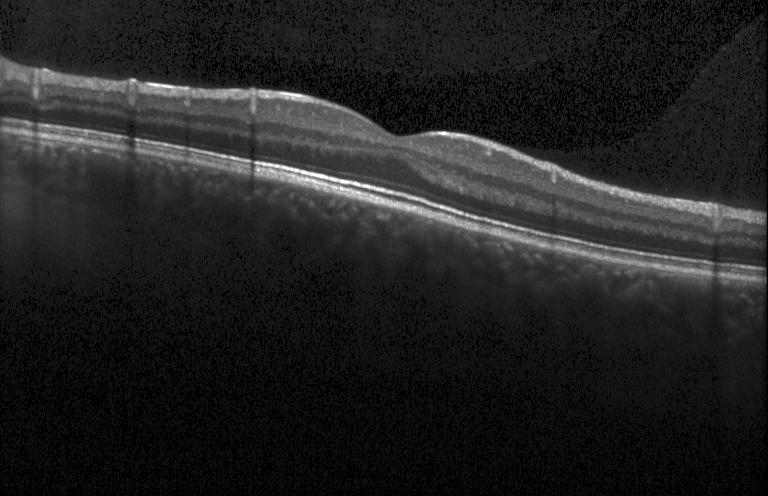
OCT line scan, spectral-domain OCT
Diagnosis: no CNV, no DME, and no drusen.